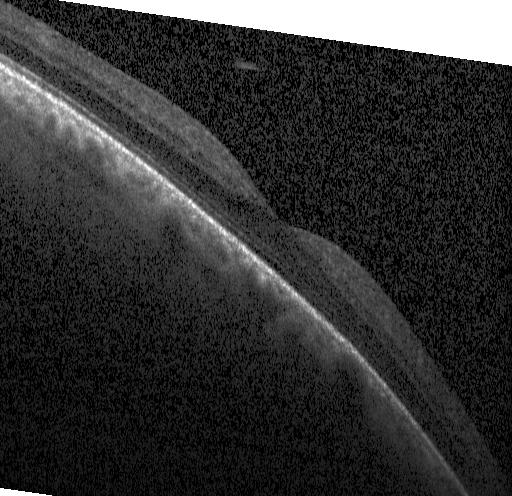

OCT B-scan — Finding: no CNV, no DME, and no drusen.